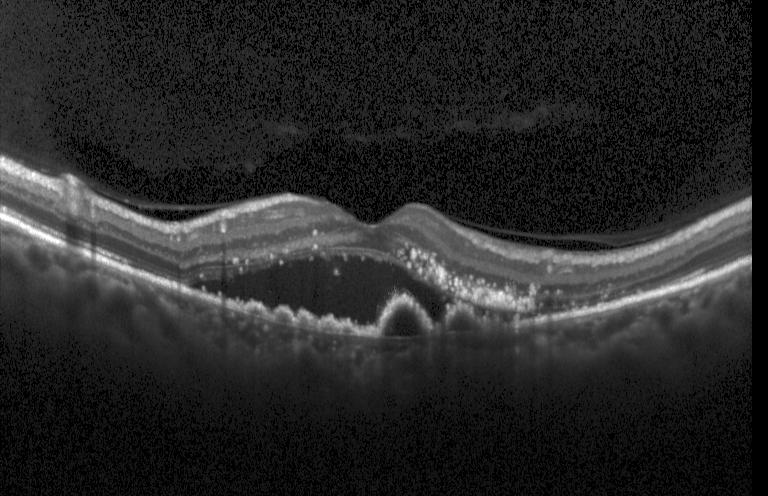

Optical coherence tomography scan; Heidelberg Spectralis OCT system; macular scan — Impression: choroidal neovascularization (CNV).